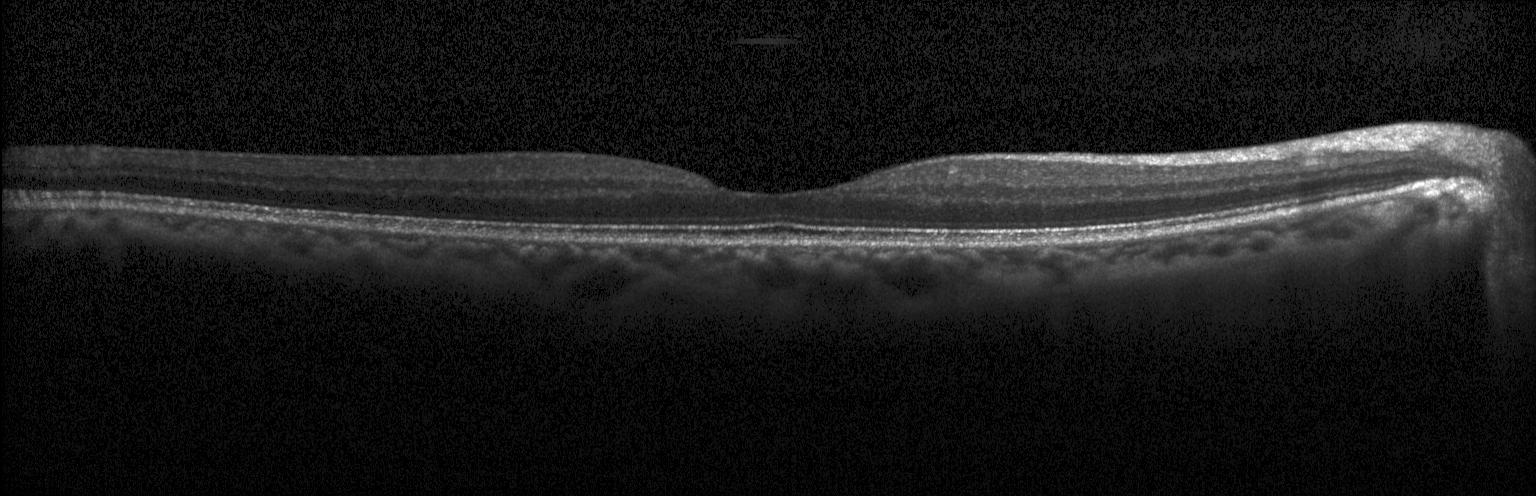
Centered on the fovea; OCT B-scan; Heidelberg Spectralis; SD-OCT. Impression: no CNV, no DME, and no drusen.